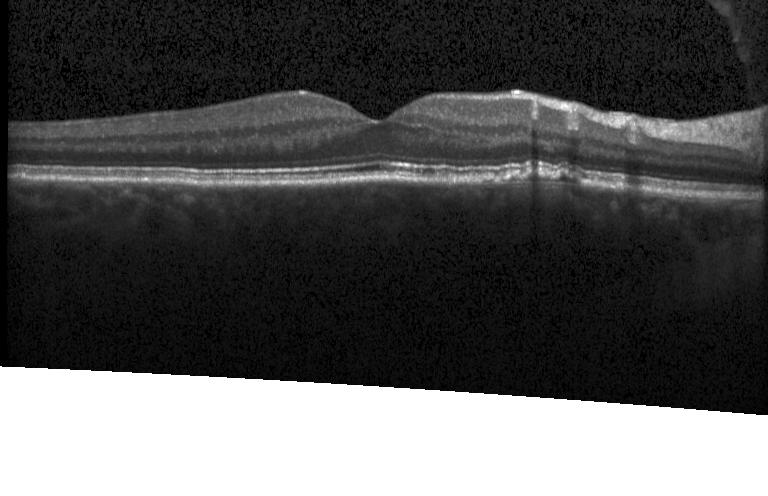
Retinal OCT B-scan. Horizontal scan through the fovea. Spectral-domain OCT — Finding: a choroidal neovascular membrane.